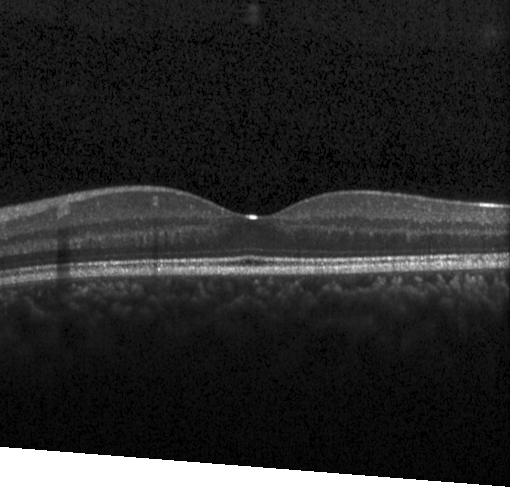 Diagnosis: neither CNV, DME, nor drusen.